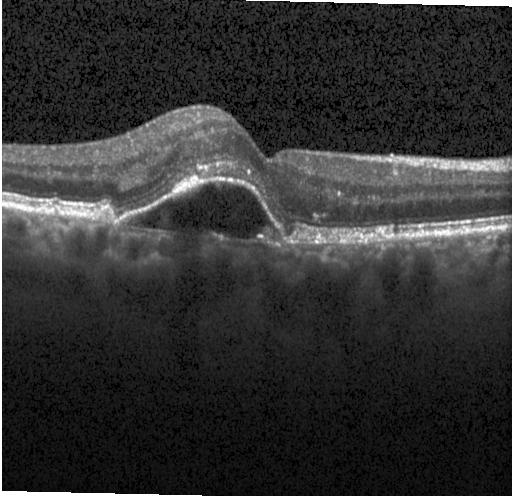

SD-OCT, optical coherence tomography scan, through the macula. Diagnosis: a choroidal neovascular membrane.